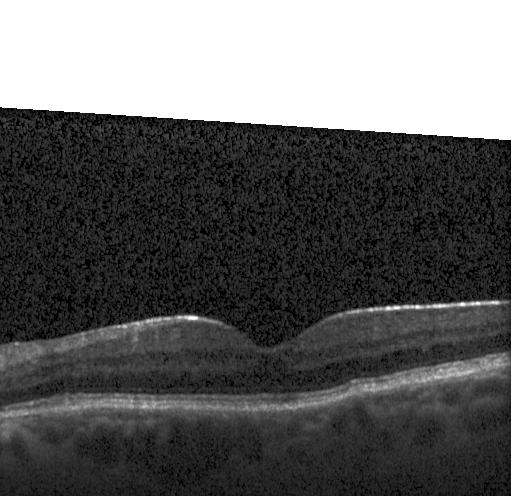
Macular OCT: no CNV, DME, or drusen.